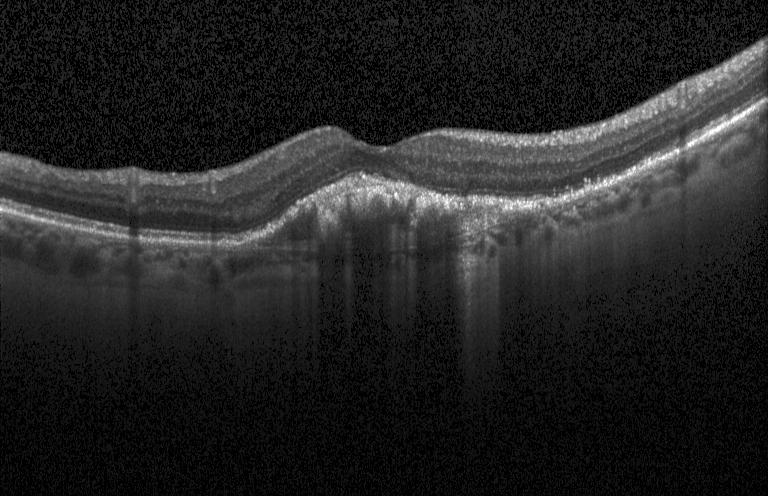
Centered on the fovea. Optical coherence tomography scan. Instrument: Heidelberg Spectralis — Impression: a choroidal neovascular membrane.